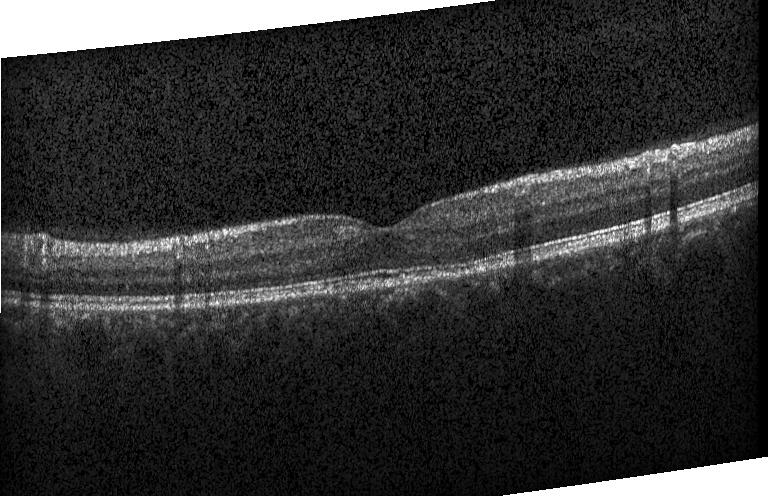 Retinal OCT B-scan. Fovea-centered. No evidence of CNV, DME, or drusen.